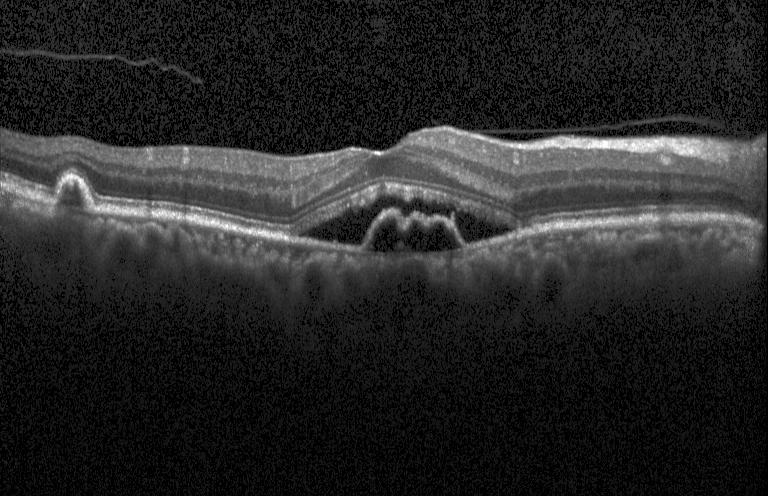
Choroidal neovascularization.